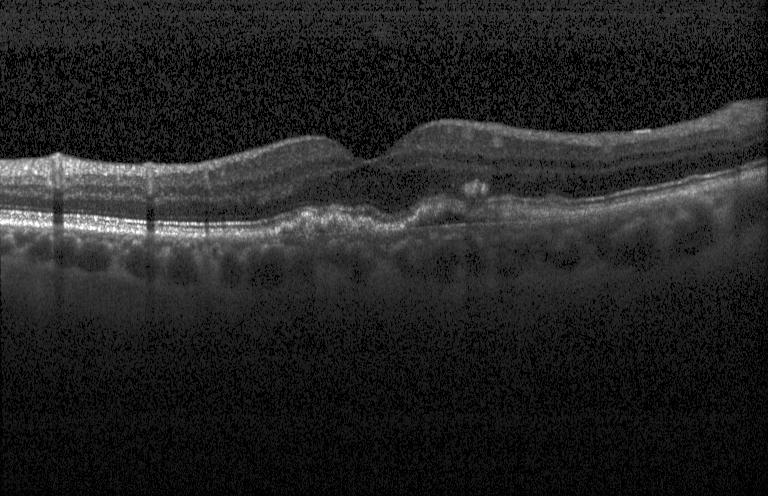
Spectral-domain optical coherence tomography; macular scan; retinal OCT cross-section. OCT finding: sub-RPE drusenoid deposits.